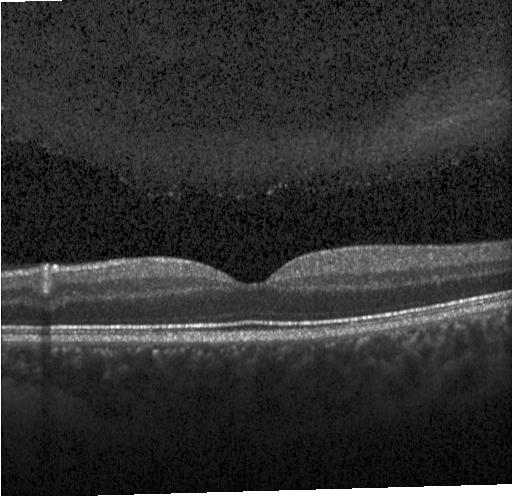
Retinal OCT B-scan.
Macular OCT: no evidence of CNV, DME, or drusen.